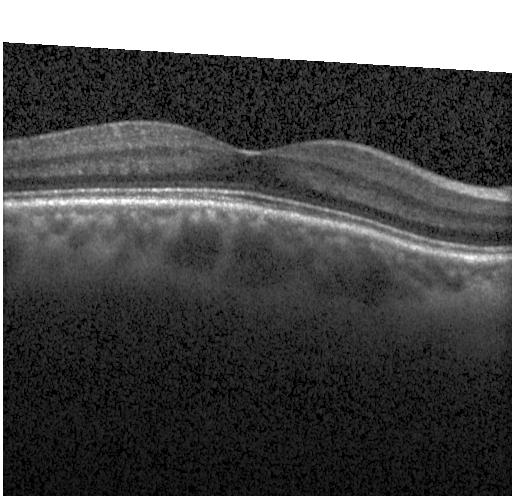
Impression: neither CNV, DME, nor drusen.